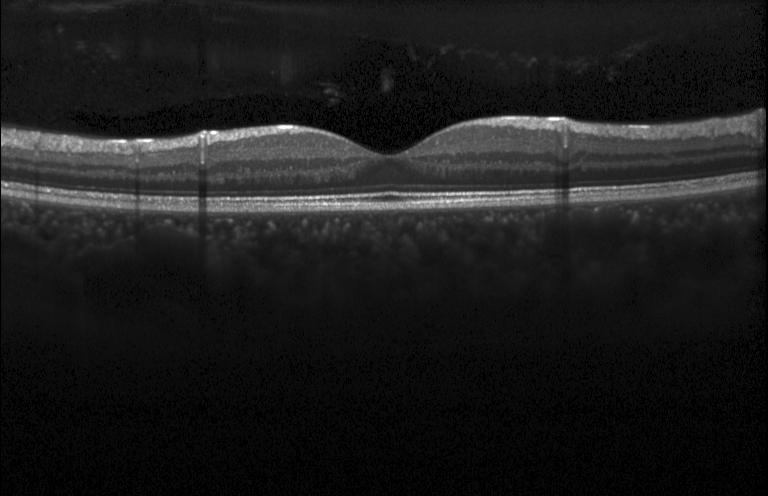

OCT finding: no choroidal neovascularization, diabetic macular edema, or drusen.